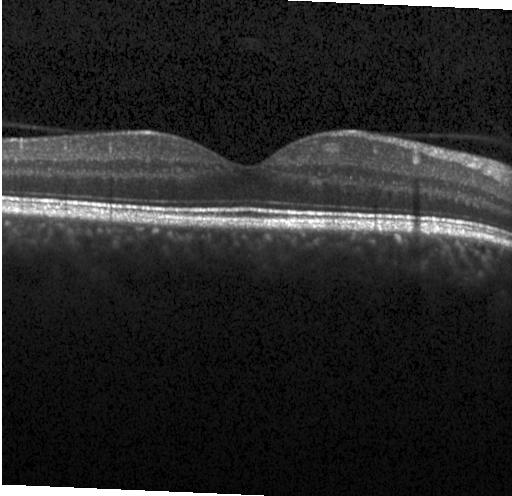
OCT line scan.
Dx: no CNV, no DME, and no drusen.